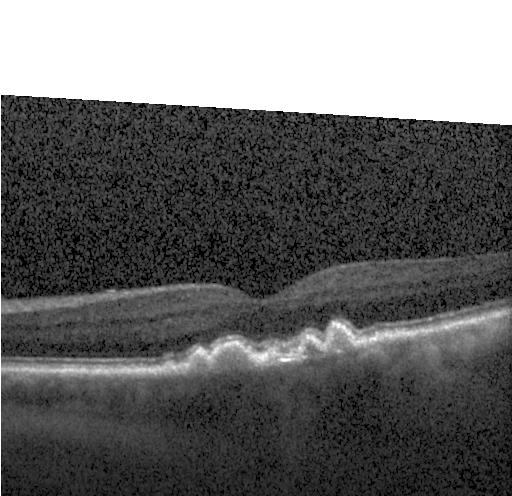
Finding: multiple drusen.